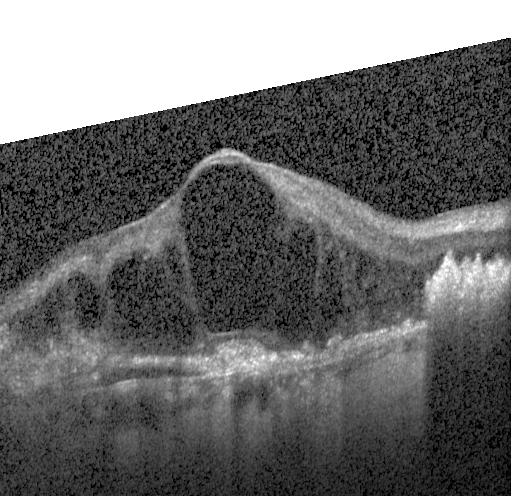
Optical coherence tomography B-scan. Centered on the fovea. Spectral-domain OCT. Instrument: Heidelberg Spectralis.
Impression: choroidal neovascularization (CNV).